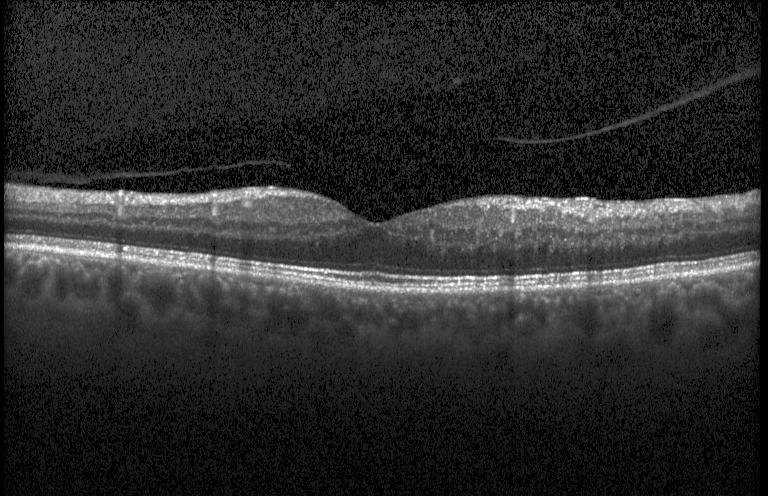

Diagnosis: no CNV, no DME, and no drusen.